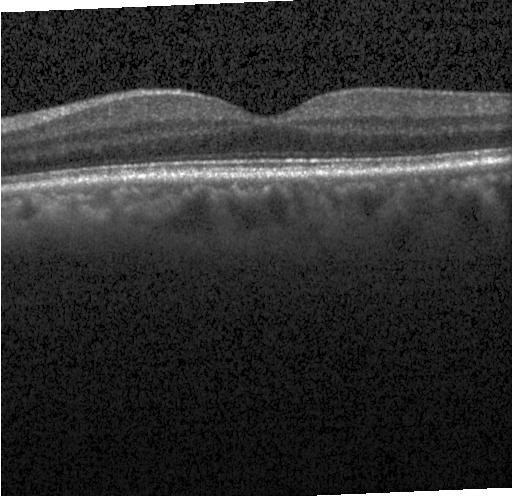 OCT line scan · spectral-domain OCT
Impression: no choroidal neovascularization, no diabetic macular edema, and no drusen.